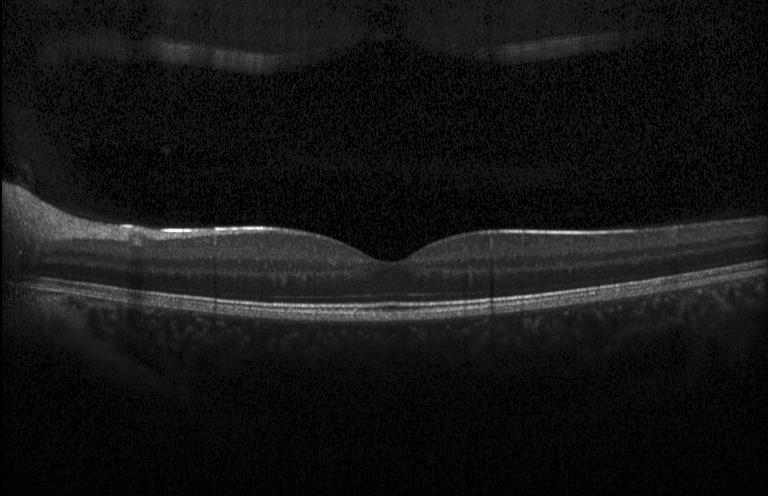 SD-OCT; horizontal scan through the fovea; acquired on a Heidelberg Spectralis; retinal OCT cross-section
Diagnosis: neither CNV, DME, nor drusen.